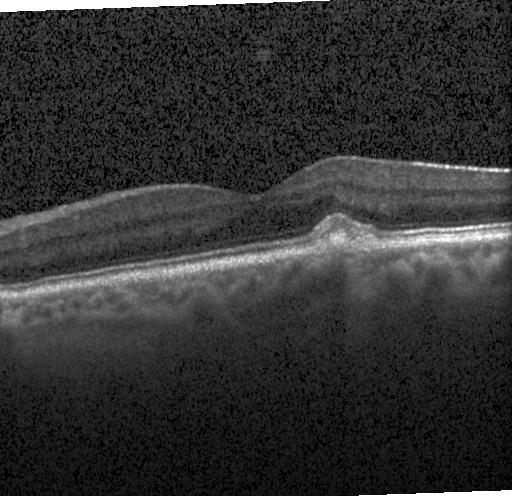
Retinal OCT B-scan · SD-OCT · through the macula. Impression: multiple drusen.